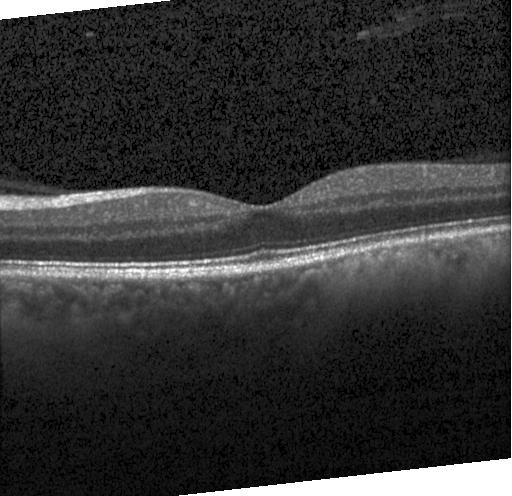
SD-OCT. Retinal OCT cross-section. Centered on the fovea.
This B-scan demonstrates no evidence of CNV, DME, or drusen.